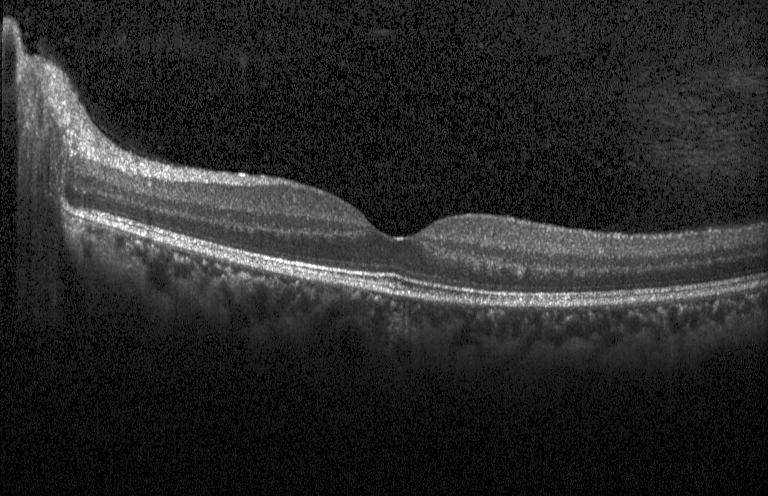 Retinal OCT cross-section. Diagnosis: no CNV, DME, or drusen.